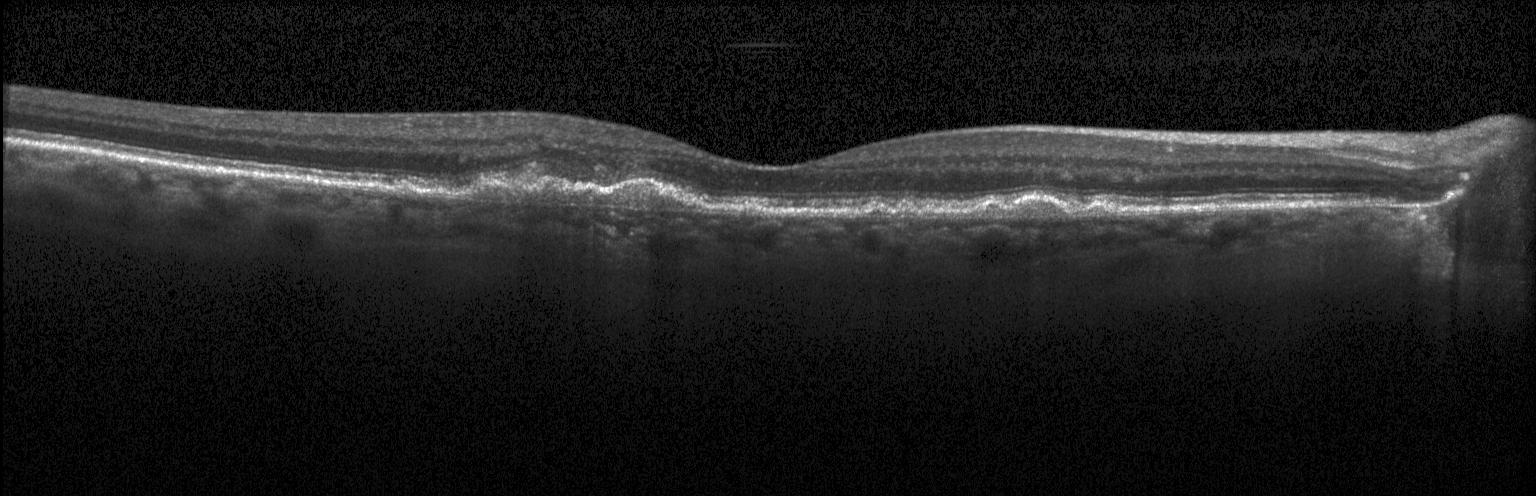

Dx: CNV.